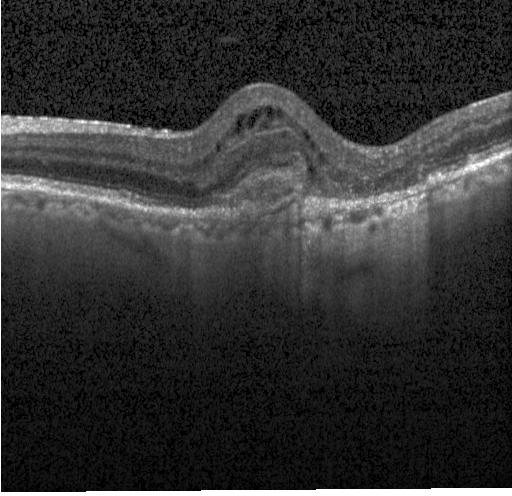
Heidelberg Spectralis, optical coherence tomography scan, fovea-centered. Macular OCT: a choroidal neovascular membrane.